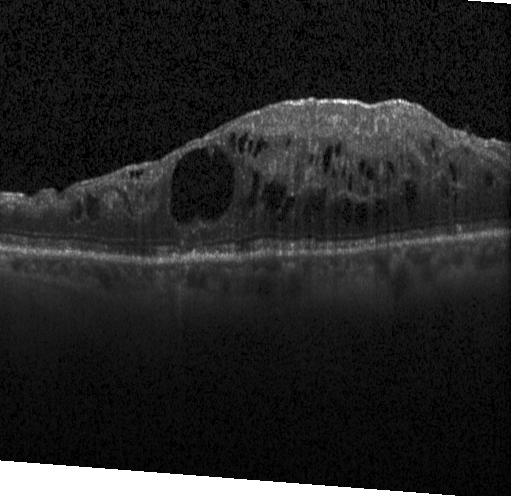

OCT line scan. Diagnosis: diabetic macular edema (DME).